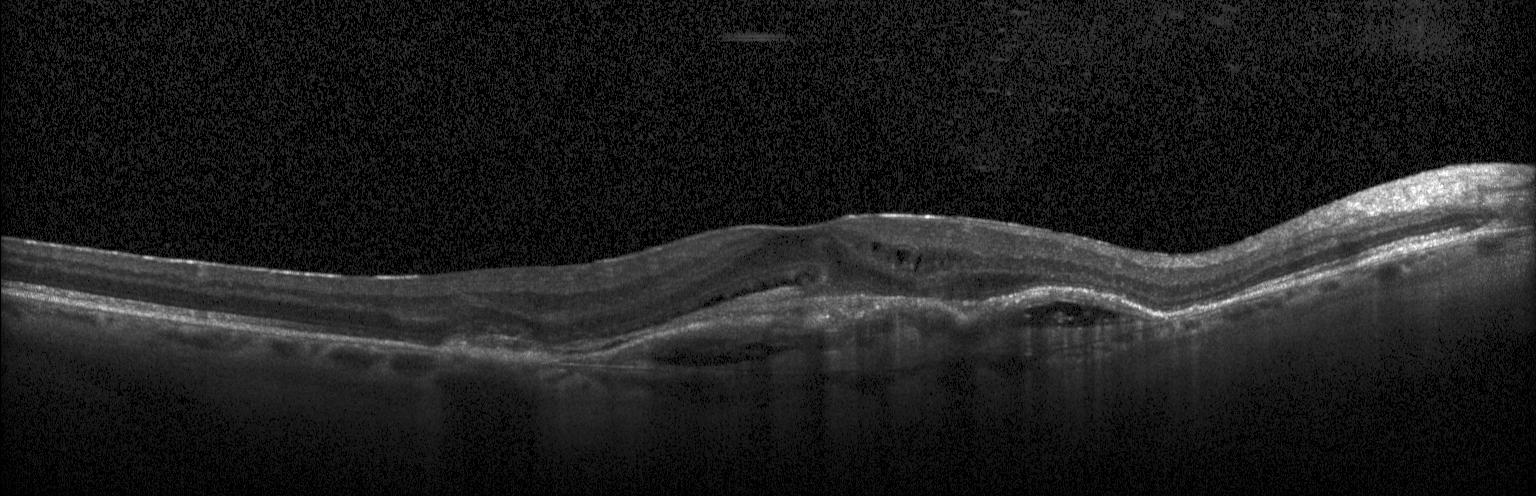
Optical coherence tomography B-scan. SD-OCT. Instrument: Heidelberg Spectralis. Impression: choroidal neovascularization (CNV).